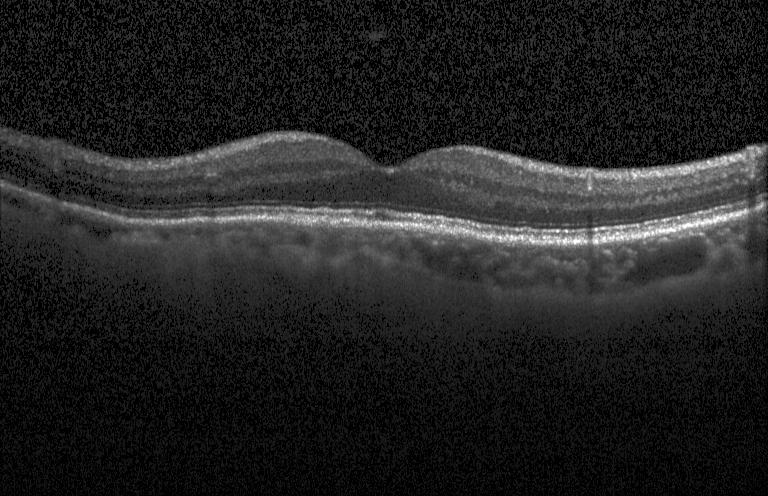
Spectral-domain optical coherence tomography; OCT B-scan
Dx: no choroidal neovascularization, no diabetic macular edema, and no drusen.